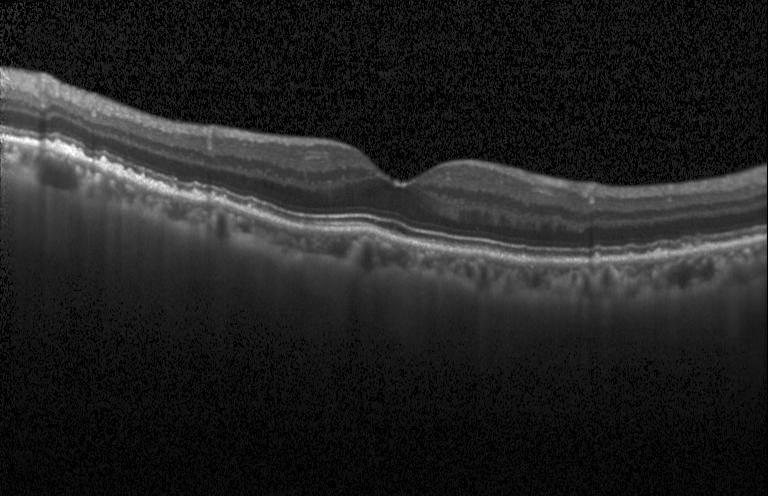

Heidelberg Spectralis · spectral-domain optical coherence tomography · retinal OCT cross-section — OCT finding: sub-RPE drusenoid deposits.